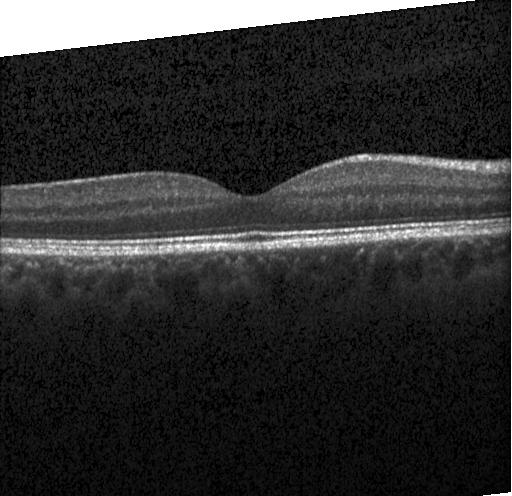 Diagnosis: neither choroidal neovascularization, diabetic macular edema, nor drusen.